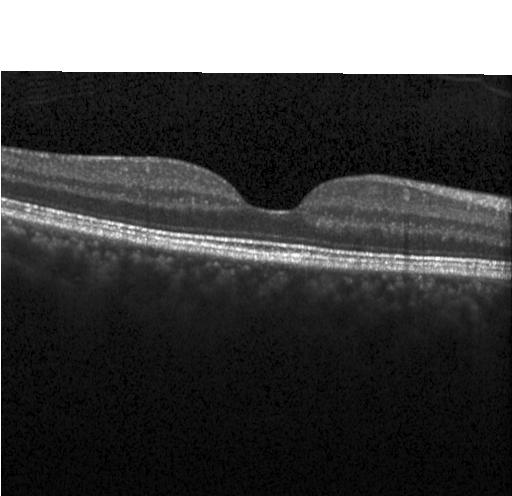 The scan shows no evidence of choroidal neovascularization, diabetic macular edema, or drusen.